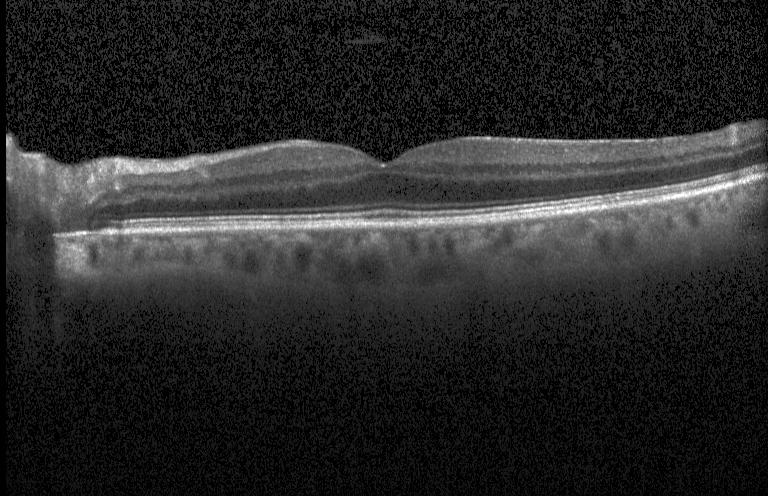 Acquired on a Heidelberg Spectralis; optical coherence tomography B-scan; spectral-domain OCT. Impression: no choroidal neovascularization, no diabetic macular edema, and no drusen.